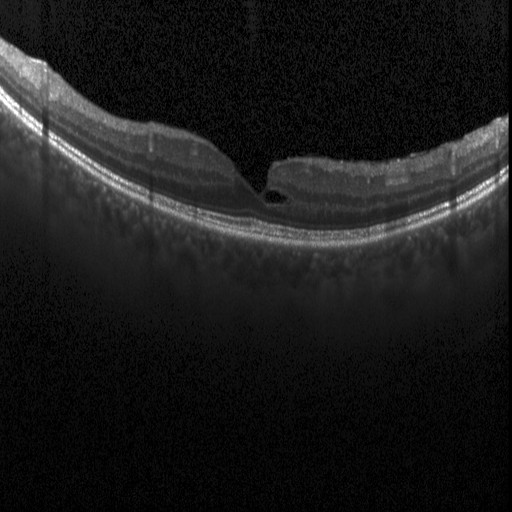

OCT line scan, macular scan
The scan shows DME.